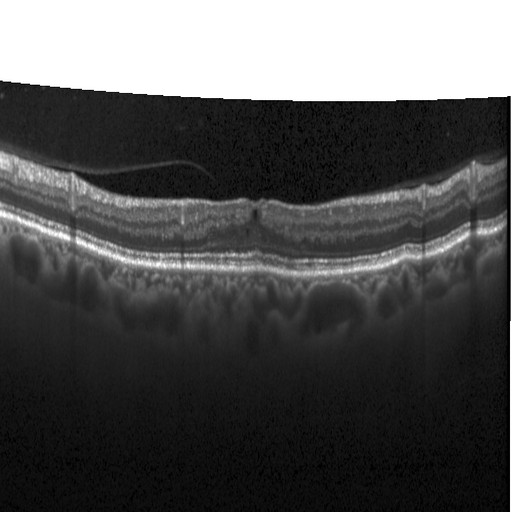
Macular OCT demonstrating diabetic macular edema (DME).